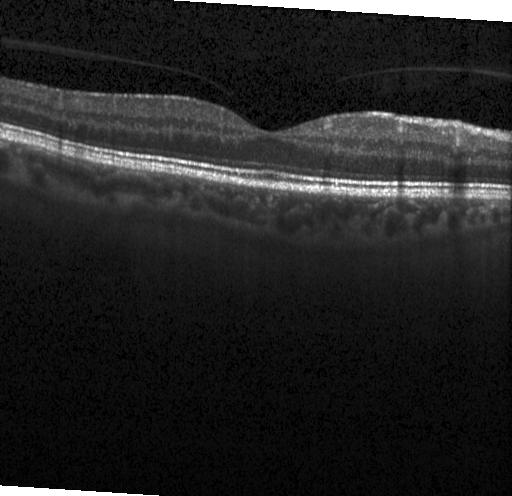

Retinal OCT B-scan. OCT finding: no choroidal neovascularization, no diabetic macular edema, and no drusen.